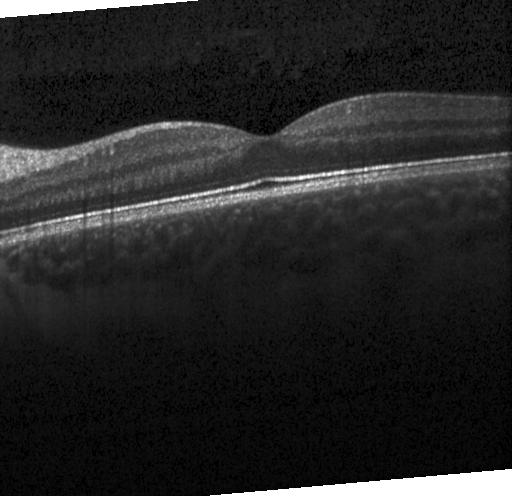
Instrument: Heidelberg Spectralis, retinal OCT cross-section, centered on the fovea, spectral-domain optical coherence tomography — Assessment: neither choroidal neovascularization, diabetic macular edema, nor drusen.